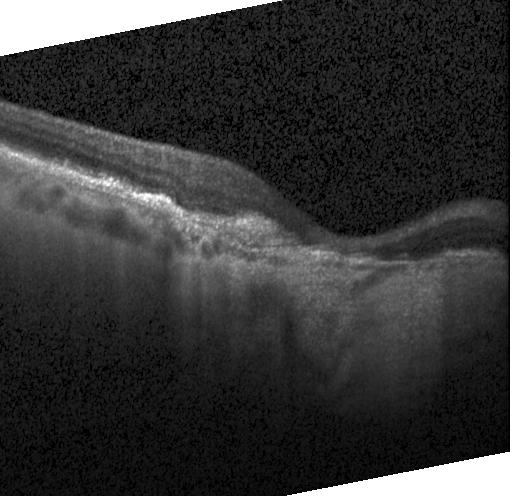

Optical coherence tomography B-scan, through the macula, Heidelberg Spectralis OCT system, spectral-domain optical coherence tomography.
Assessment: choroidal neovascularization.